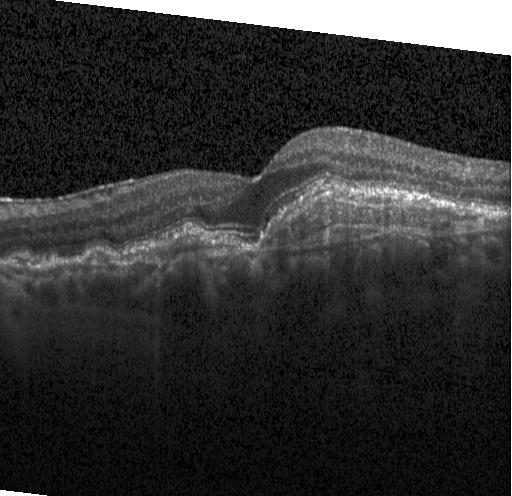

Retinal OCT cross-section, fovea-centered — Impression: a choroidal neovascular membrane.